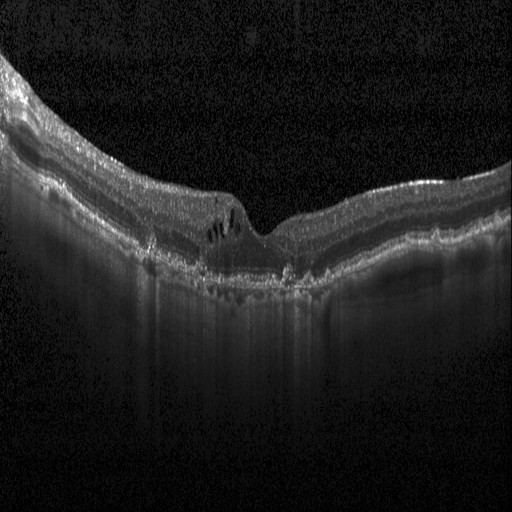 Retinal OCT cross-section. SD-OCT. Centered on the fovea — Finding: DME.